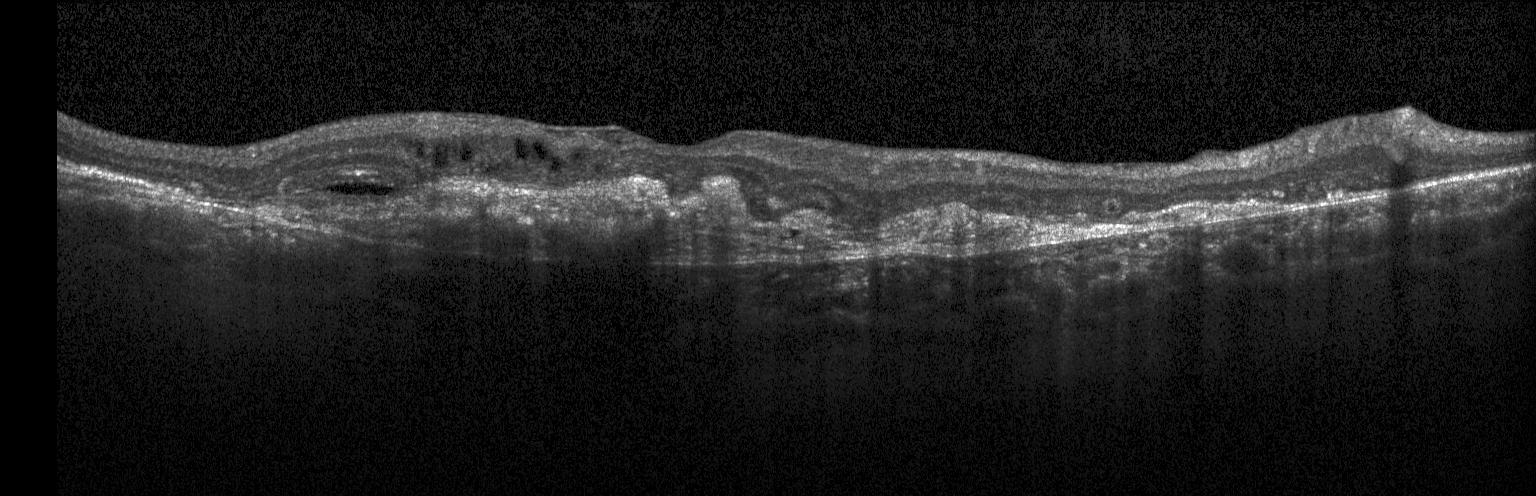
Macular OCT: choroidal neovascularization.